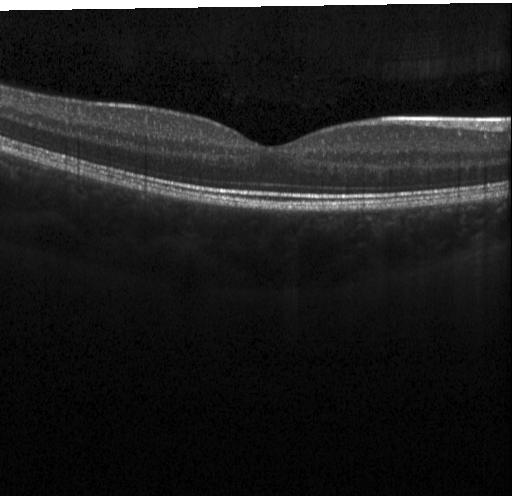 Impression: neither CNV, DME, nor drusen.